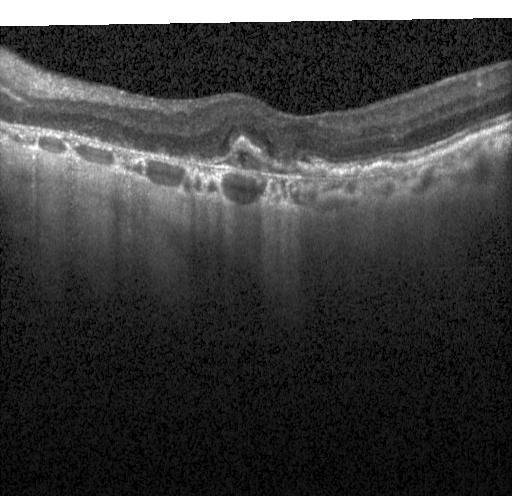

Centered on the fovea · spectral-domain optical coherence tomography · Heidelberg Spectralis OCT system · retinal OCT B-scan
This B-scan demonstrates a choroidal neovascular membrane.